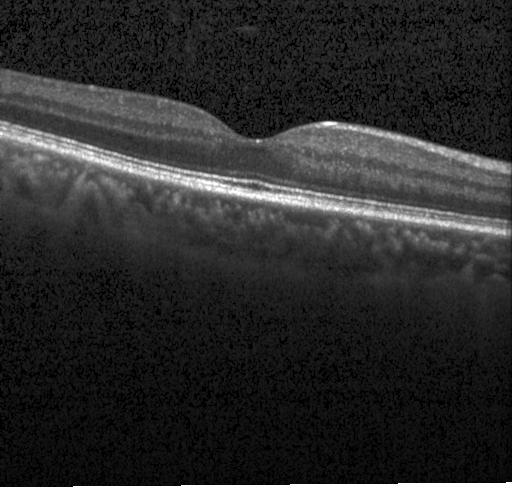
Optical coherence tomography B-scan
Finding: no choroidal neovascularization, no diabetic macular edema, and no drusen.